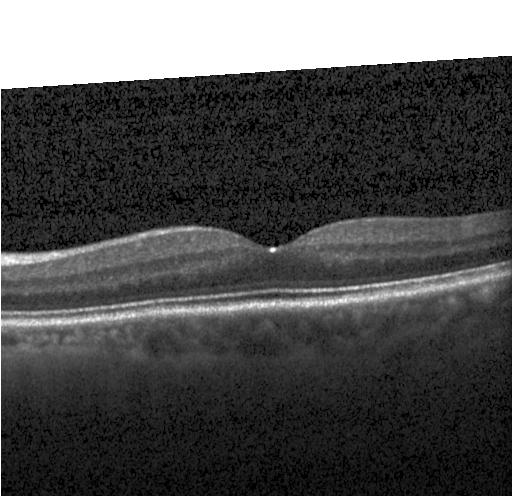 Instrument: Heidelberg Spectralis. Optical coherence tomography scan. SD-OCT. Horizontal scan through the fovea — Finding: neither choroidal neovascularization, diabetic macular edema, nor drusen.